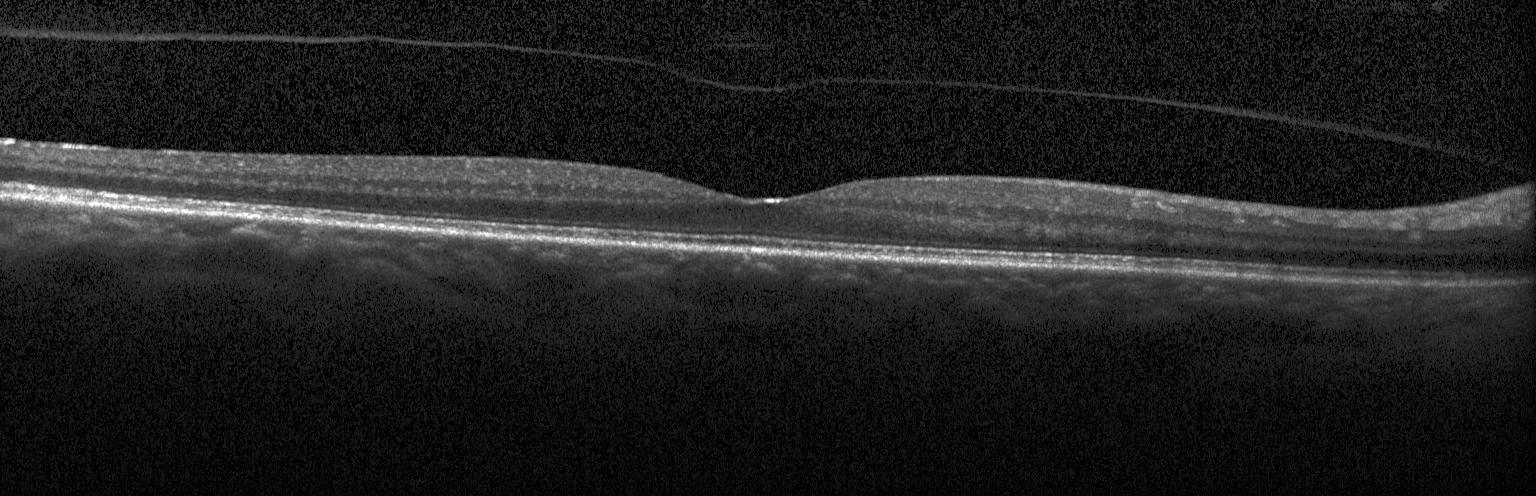

Heidelberg Spectralis, optical coherence tomography B-scan — Macular OCT: neither choroidal neovascularization, diabetic macular edema, nor drusen.